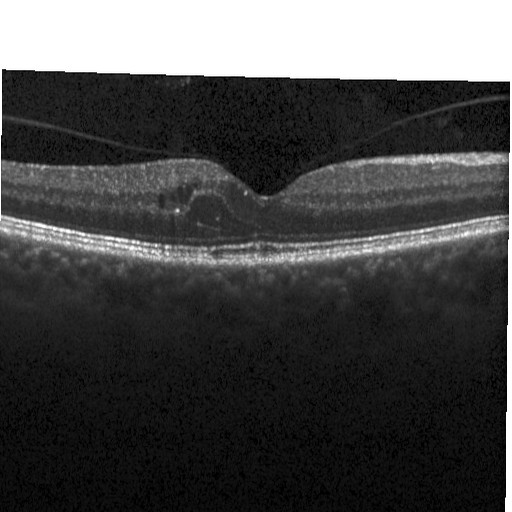 Impression: diabetic macular edema (DME).